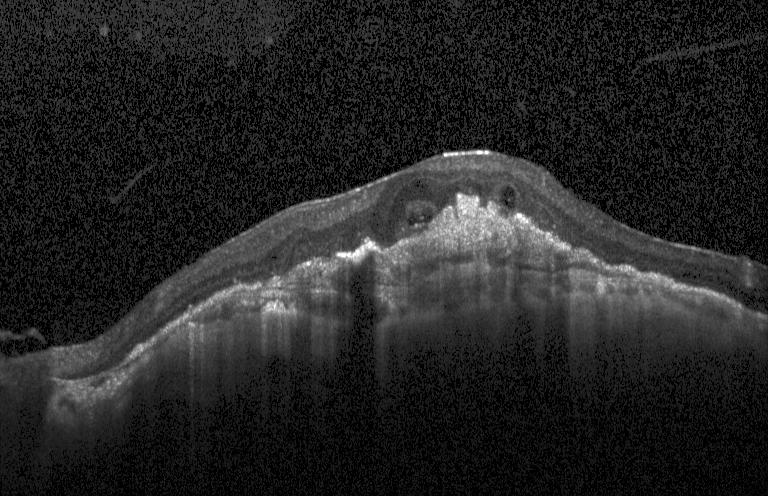

Heidelberg Spectralis; OCT B-scan
Macular OCT: CNV.